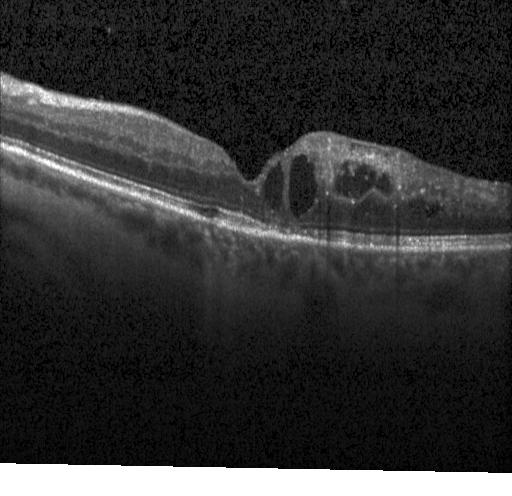
OCT B-scan showing diabetic macular edema (DME).